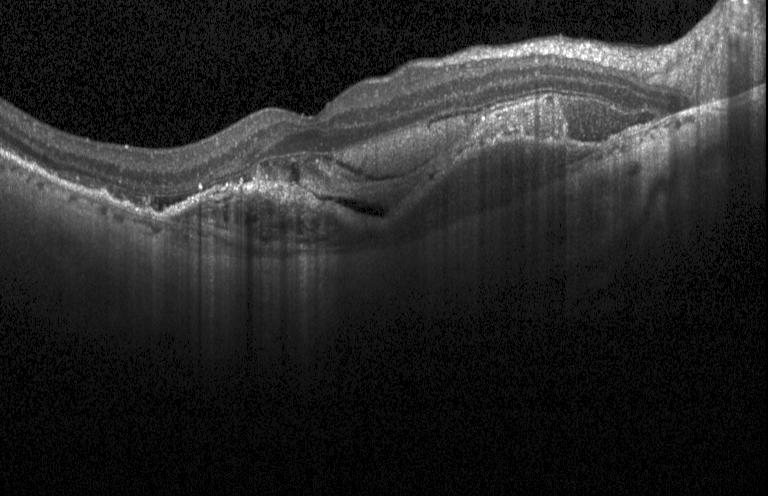
Finding: choroidal neovascularization.